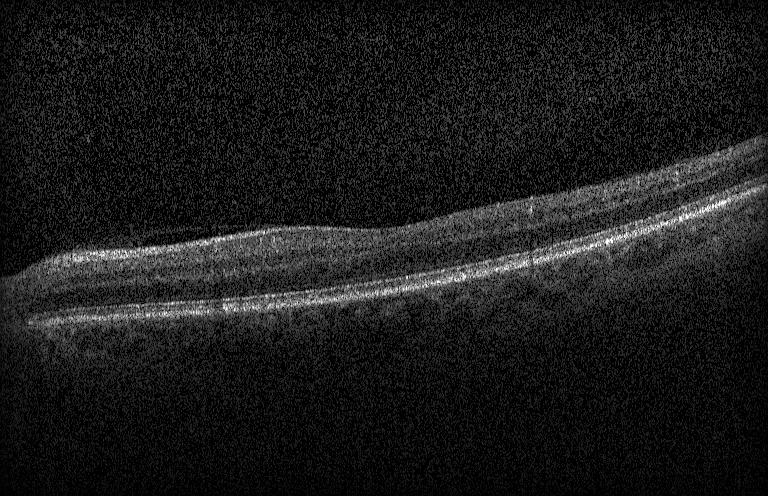 OCT B-scan — Impression: no evidence of choroidal neovascularization, diabetic macular edema, or drusen.